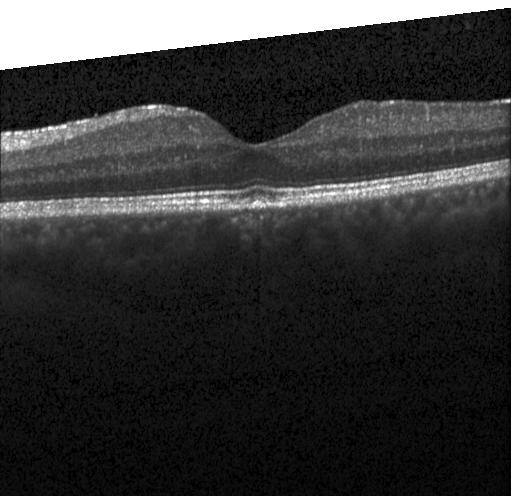
OCT line scan. Horizontal scan through the fovea. Spectral-domain optical coherence tomography. Instrument: Heidelberg Spectralis.
Finding: neither choroidal neovascularization, diabetic macular edema, nor drusen.